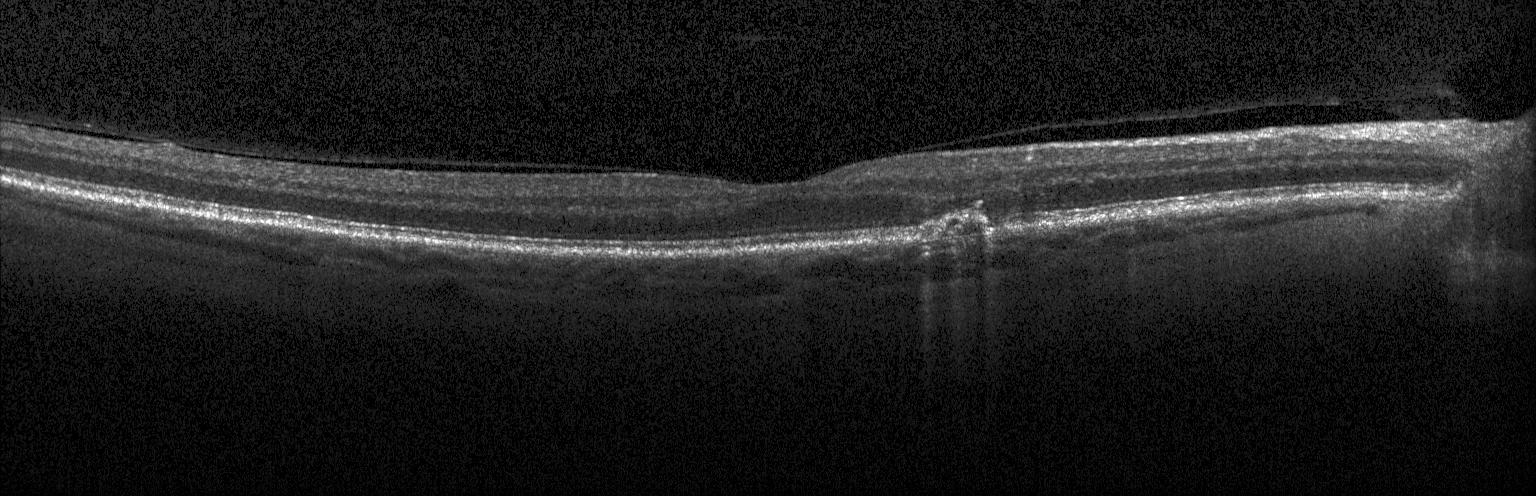

Optical coherence tomography B-scan · instrument: Heidelberg Spectralis · through the macula.
This B-scan demonstrates drusen.